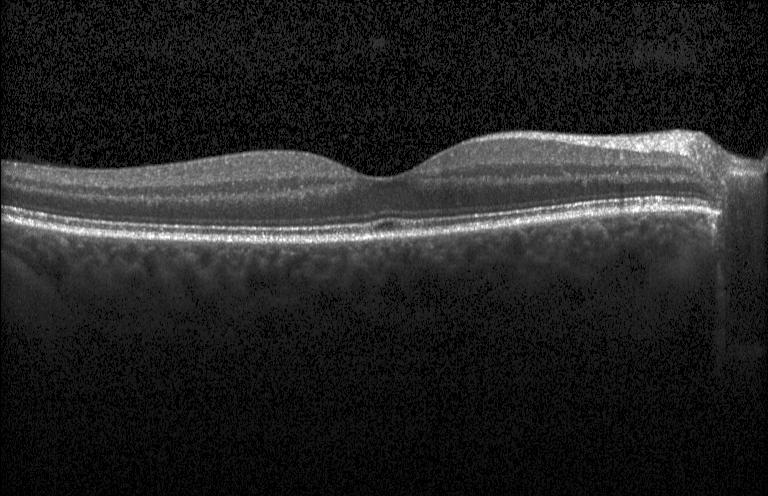

Retinal OCT cross-section, centered on the fovea, spectral-domain OCT, Heidelberg Spectralis
Dx: neither choroidal neovascularization, diabetic macular edema, nor drusen.